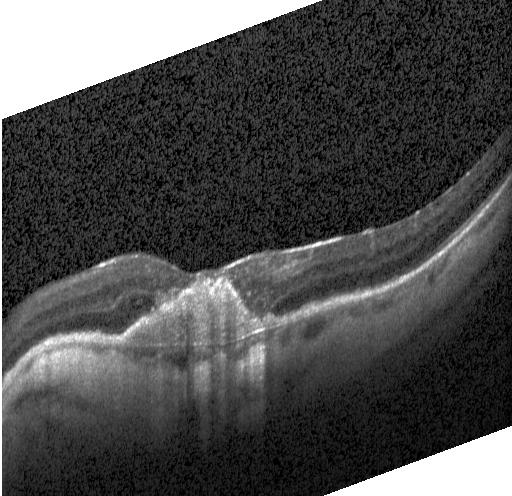

Spectral-domain optical coherence tomography · optical coherence tomography scan · Heidelberg Spectralis OCT system.
This B-scan demonstrates a choroidal neovascular membrane.